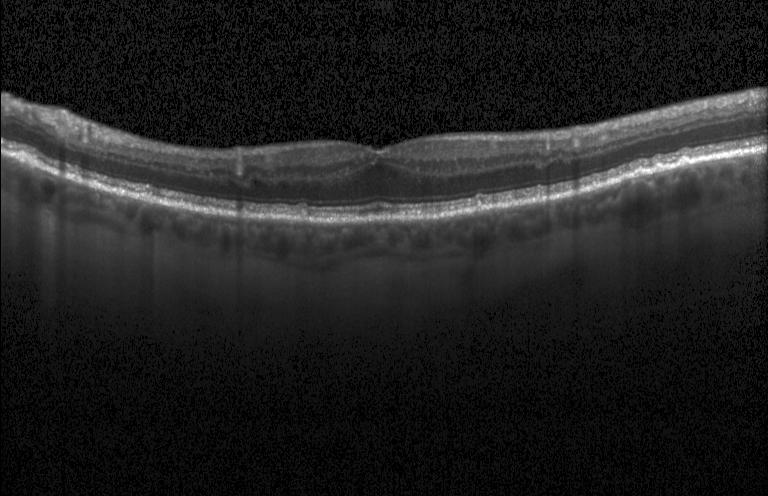 Macular OCT demonstrating sub-RPE drusenoid deposits.